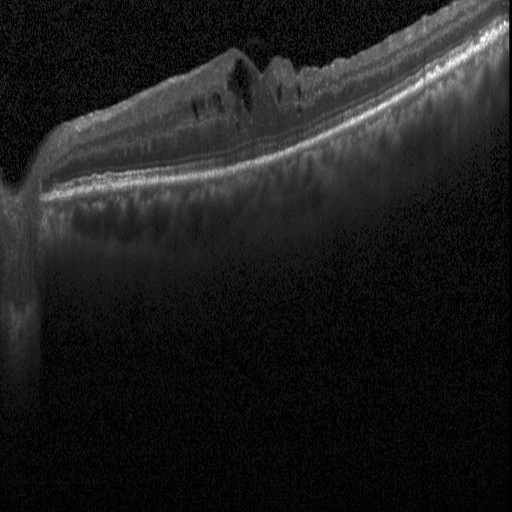
OCT finding: diabetic macular edema.